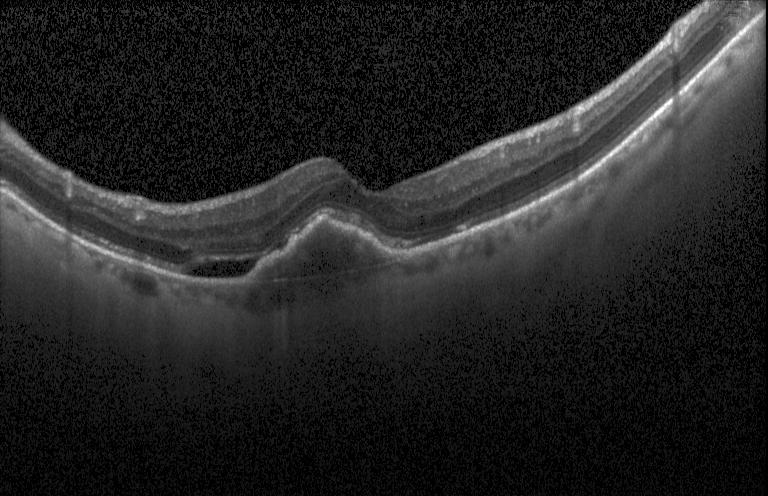
OCT B-scan, macular scan, spectral-domain OCT
The scan shows a choroidal neovascular membrane.